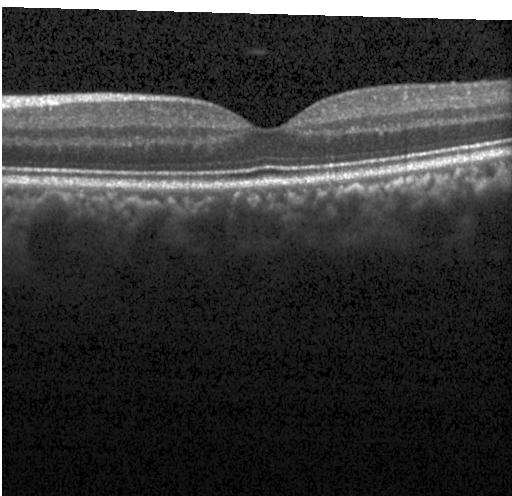
Optical coherence tomography scan, spectral-domain OCT. Finding: no CNV, DME, or drusen.